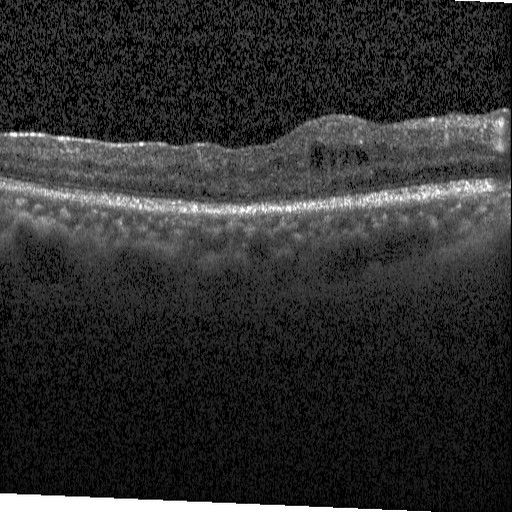
Spectral-domain optical coherence tomography; OCT B-scan. Macular OCT: diabetic macular edema (DME).